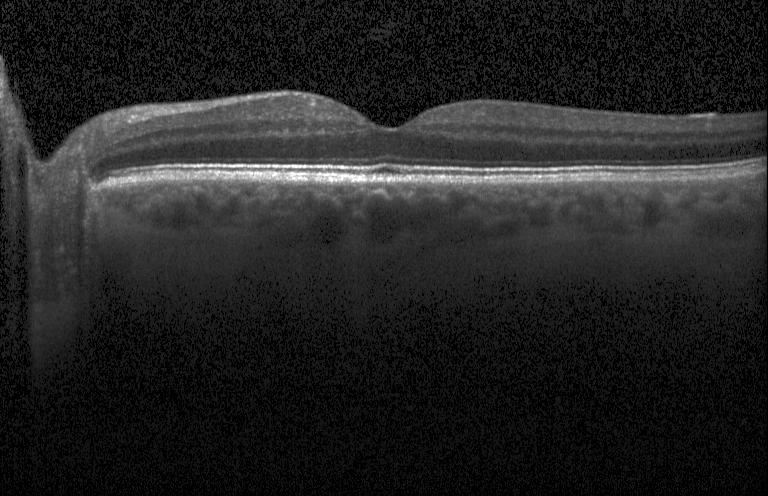
The scan shows no CNV, no DME, and no drusen.